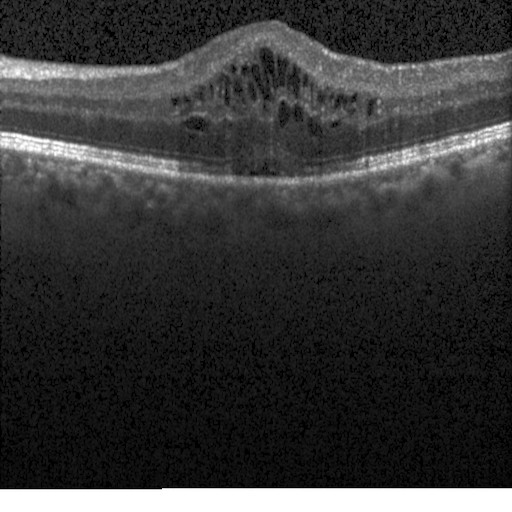 Optical coherence tomography scan, Heidelberg Spectralis OCT system, macular scan. Assessment: diabetic macular edema.